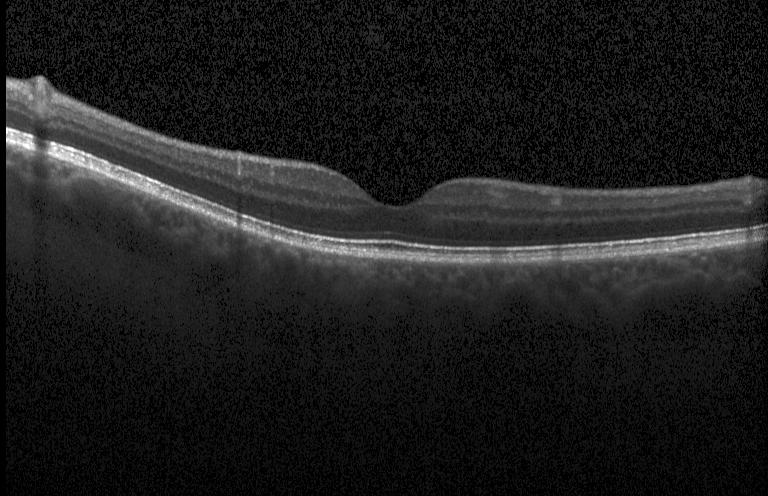

Optical coherence tomography B-scan · spectral-domain optical coherence tomography · Heidelberg Spectralis · horizontal scan through the fovea.
OCT finding: neither choroidal neovascularization, diabetic macular edema, nor drusen.